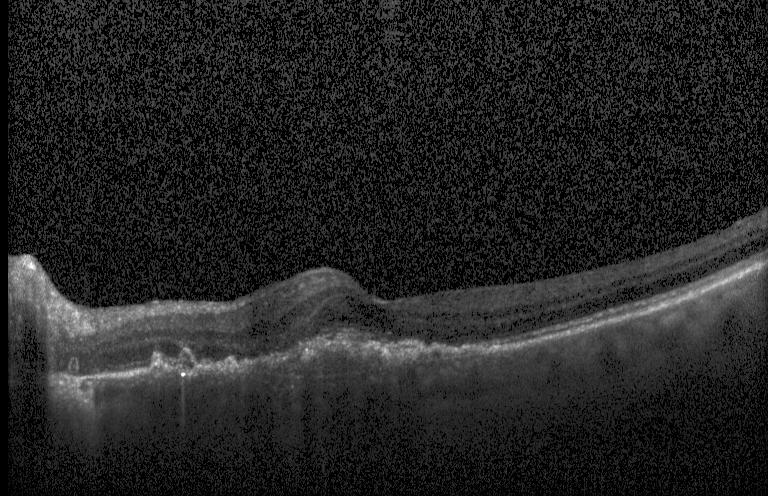
Spectral-domain OCT, optical coherence tomography scan
Assessment: a choroidal neovascular membrane.